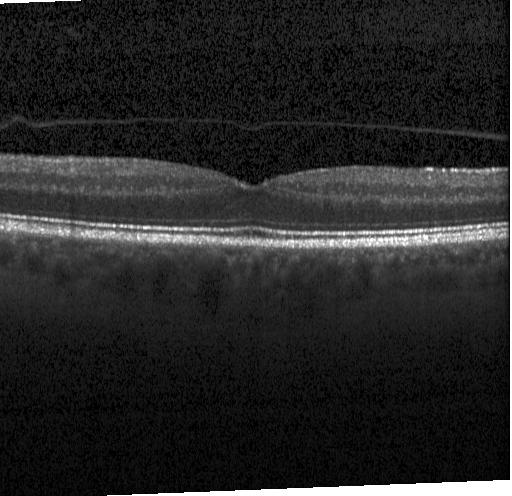
Diagnosis: no choroidal neovascularization, diabetic macular edema, or drusen.